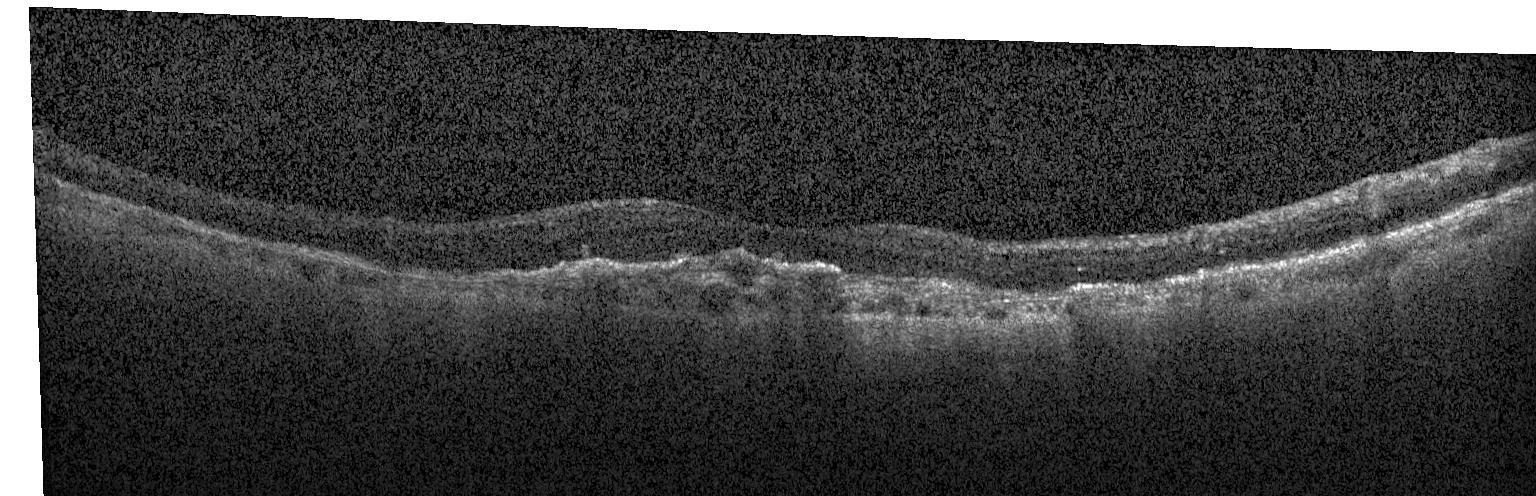

OCT line scan — Dx: CNV.